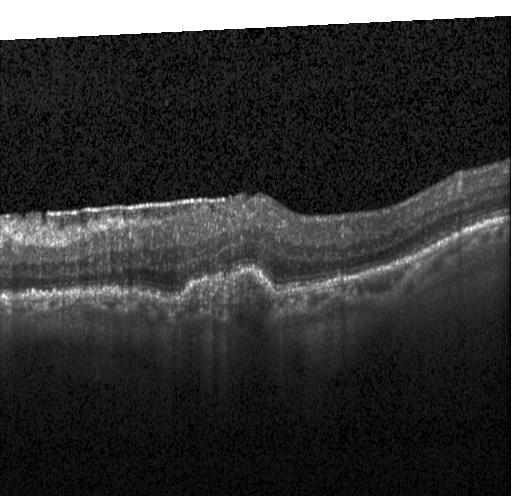 Optical coherence tomography B-scan · Heidelberg Spectralis OCT system — Impression: a choroidal neovascular membrane.